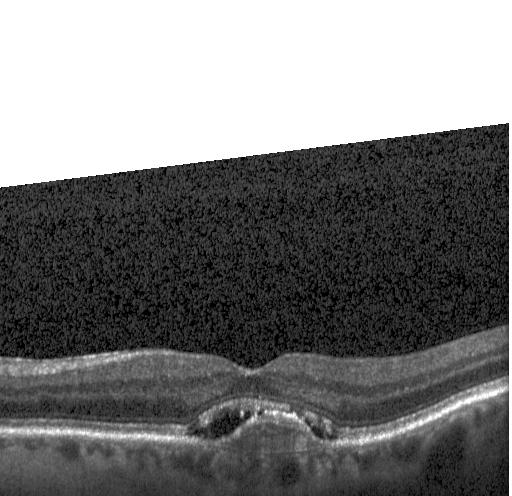

OCT line scan — Impression: a choroidal neovascular membrane.